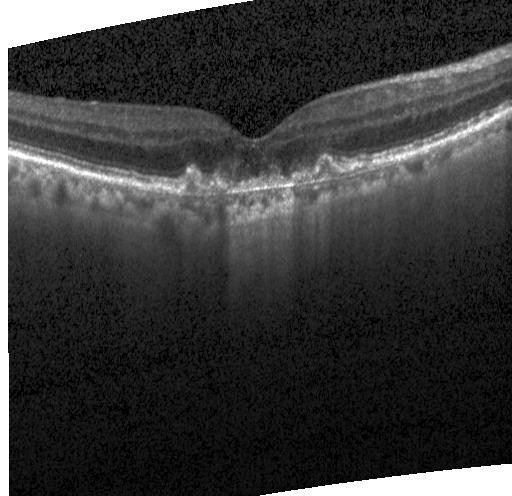

Horizontal scan through the fovea, SD-OCT, optical coherence tomography scan.
Dx: choroidal neovascularization (CNV).